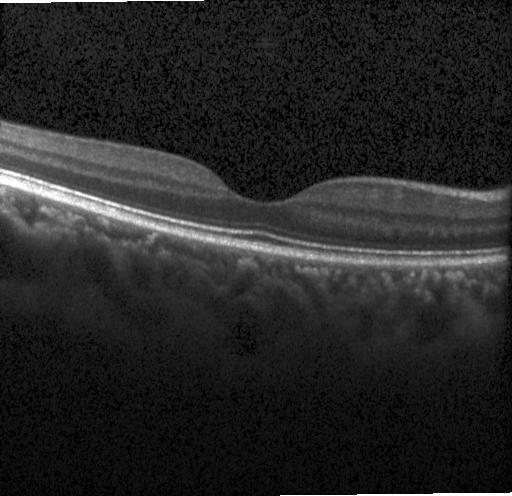 Finding: neither choroidal neovascularization, diabetic macular edema, nor drusen.